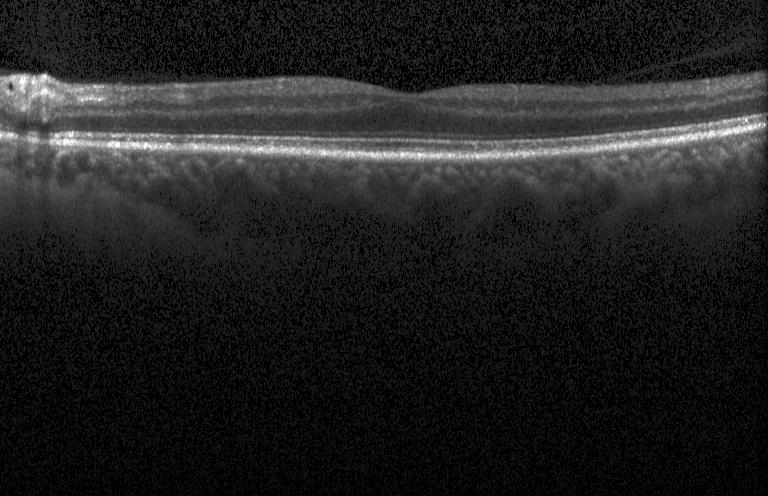
Spectral-domain optical coherence tomography, through the macula, optical coherence tomography B-scan, acquired on a Heidelberg Spectralis.
Impression: no CNV, DME, or drusen.